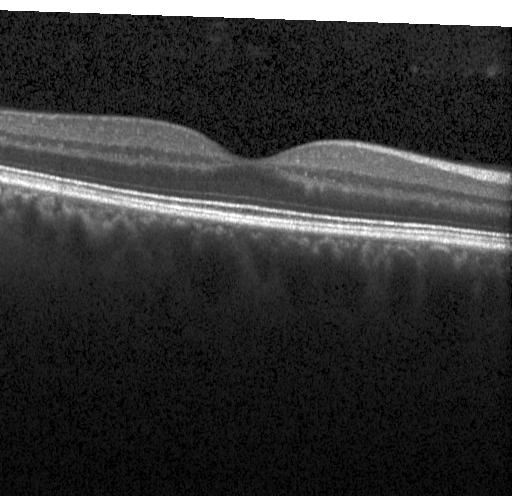
Retinal OCT cross-section. Spectral-domain optical coherence tomography. Through the macula. Heidelberg Spectralis OCT system — Finding: no choroidal neovascularization, no diabetic macular edema, and no drusen.